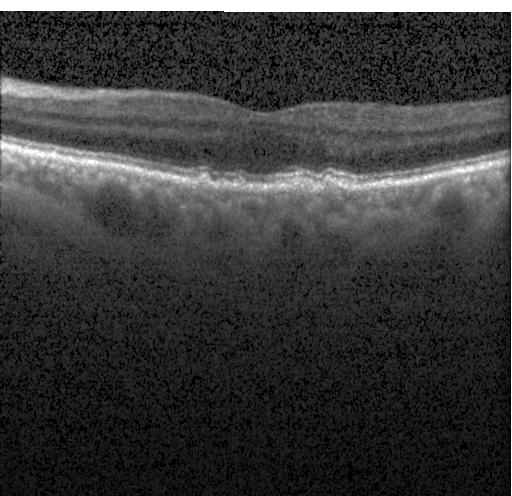
Macular scan. Heidelberg Spectralis OCT system. Spectral-domain optical coherence tomography. Retinal OCT cross-section
Finding: sub-RPE drusenoid deposits.